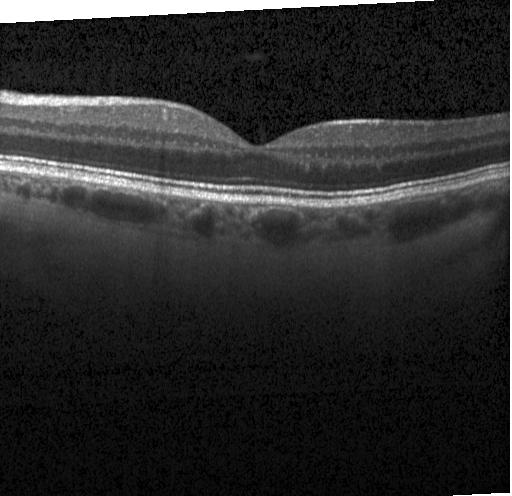
Retinal OCT cross-section; Heidelberg Spectralis; spectral-domain OCT; through the macula.
No CNV, DME, or drusen.